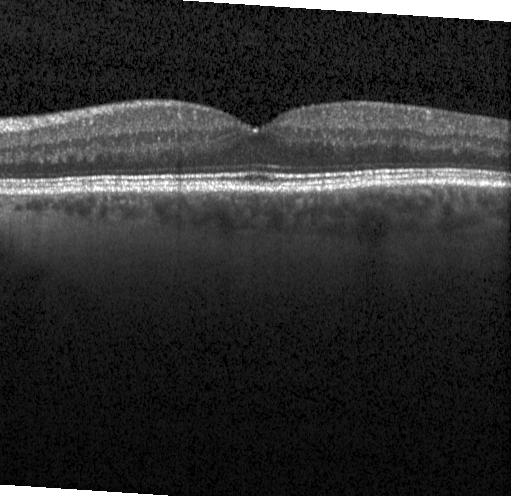 SD-OCT. Optical coherence tomography scan
No choroidal neovascularization, diabetic macular edema, or drusen.